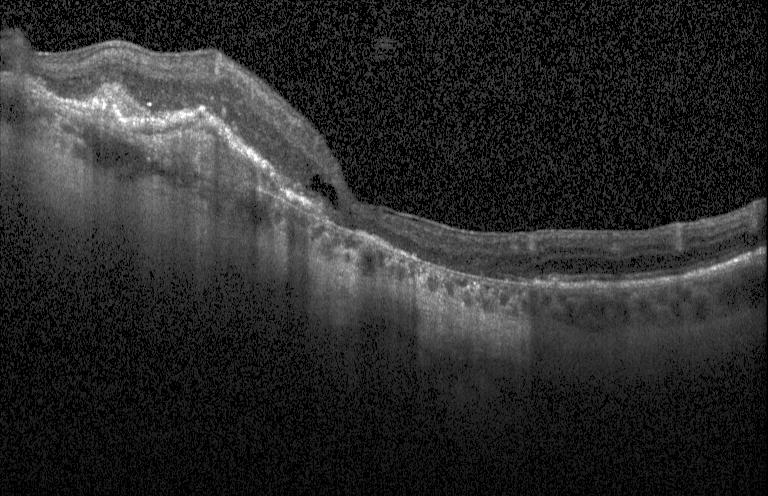
Heidelberg Spectralis OCT system · SD-OCT · through the macula · retinal OCT cross-section. Dx: a choroidal neovascular membrane.